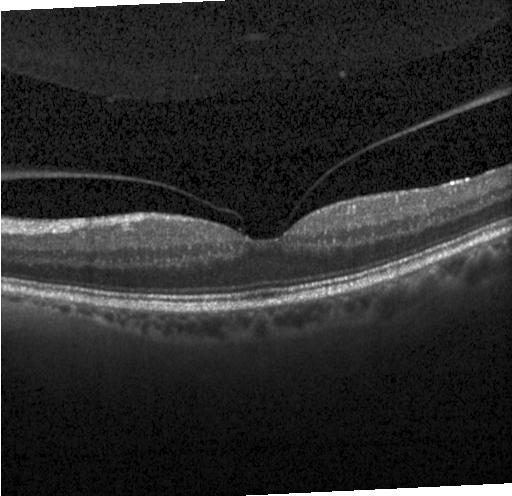

Fovea-centered, spectral-domain optical coherence tomography, OCT line scan — OCT finding: no CNV, no DME, and no drusen.